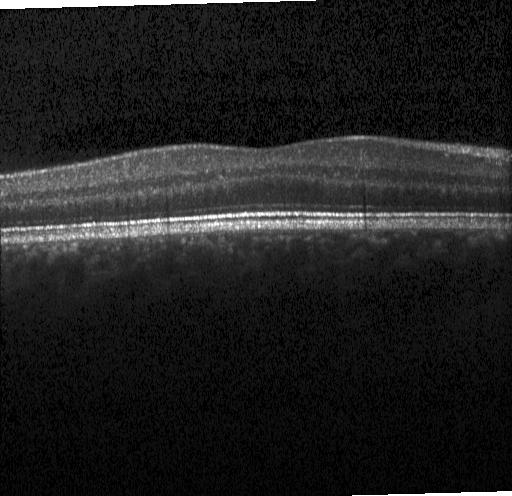 SD-OCT · acquired on a Heidelberg Spectralis · horizontal scan through the fovea · OCT B-scan
This B-scan demonstrates neither choroidal neovascularization, diabetic macular edema, nor drusen.